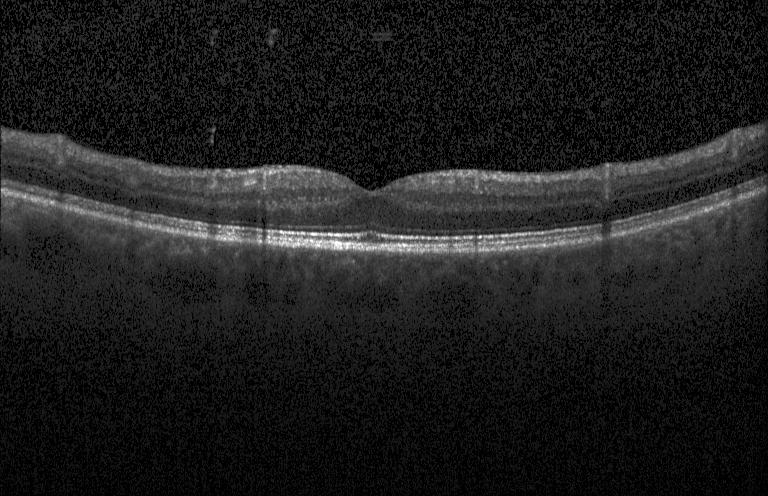 Macular OCT demonstrating no choroidal neovascularization, no diabetic macular edema, and no drusen.